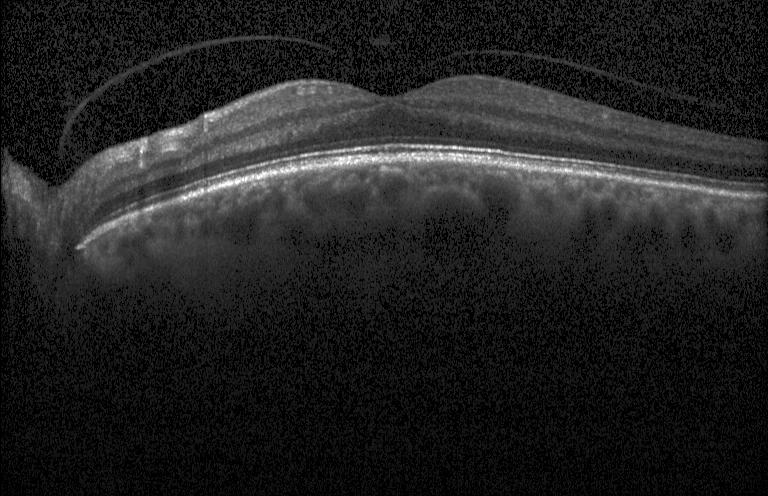 Macular OCT: no evidence of CNV, DME, or drusen.